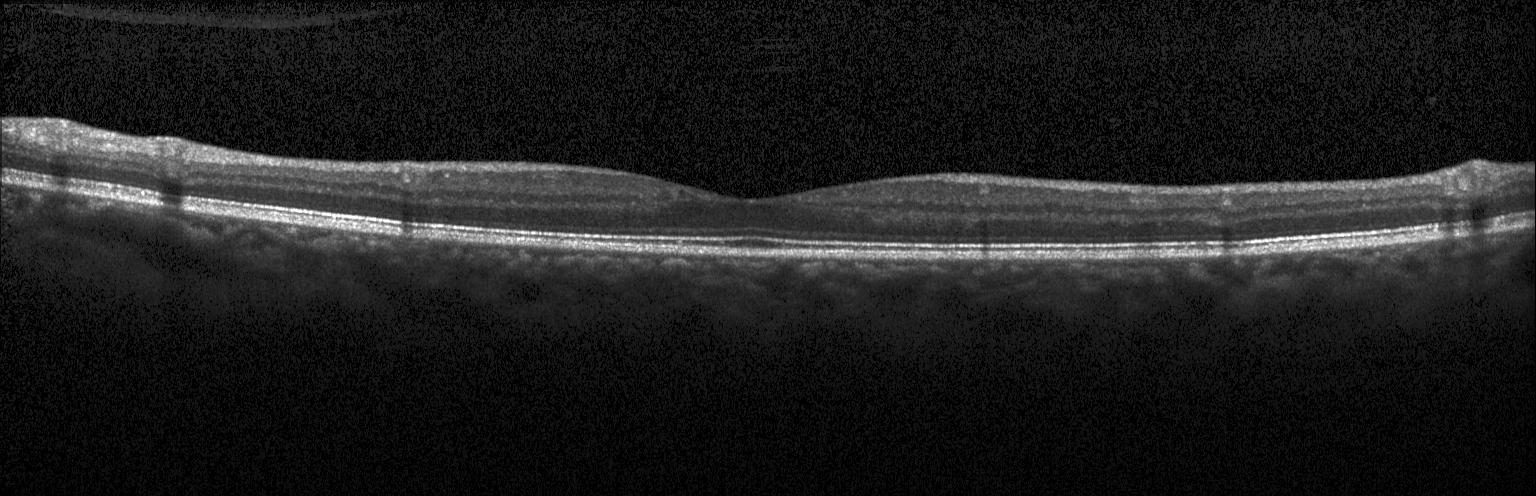 SD-OCT; centered on the fovea; optical coherence tomography scan. Macular OCT: no CNV, no DME, and no drusen.